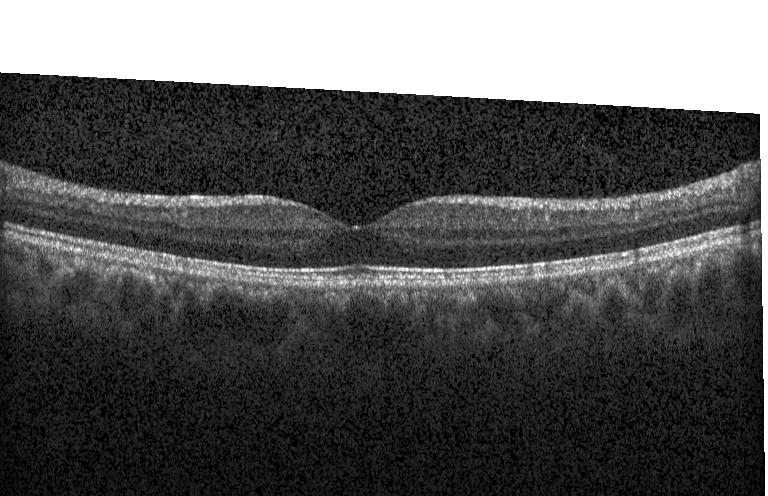

OCT finding: neither choroidal neovascularization, diabetic macular edema, nor drusen.